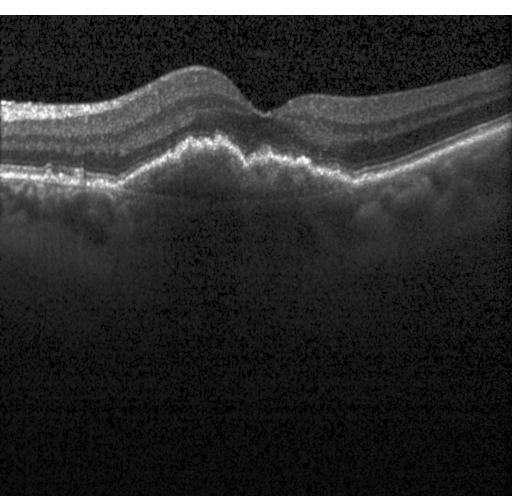 Macular OCT demonstrating choroidal neovascularization.